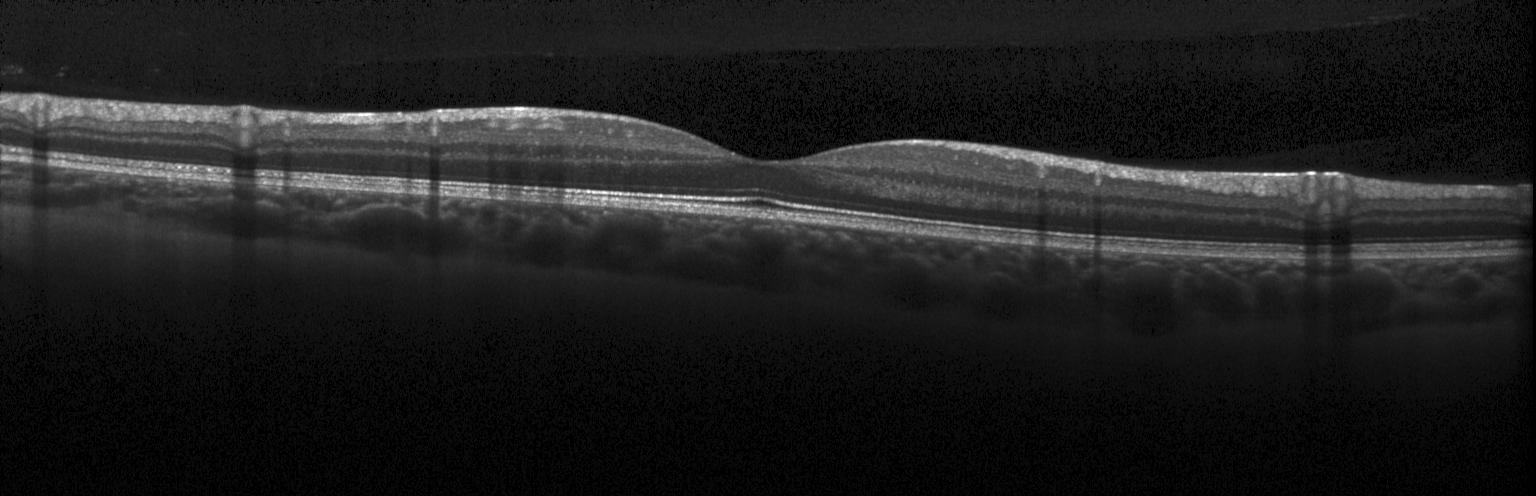
Diagnosis: no choroidal neovascularization, no diabetic macular edema, and no drusen.